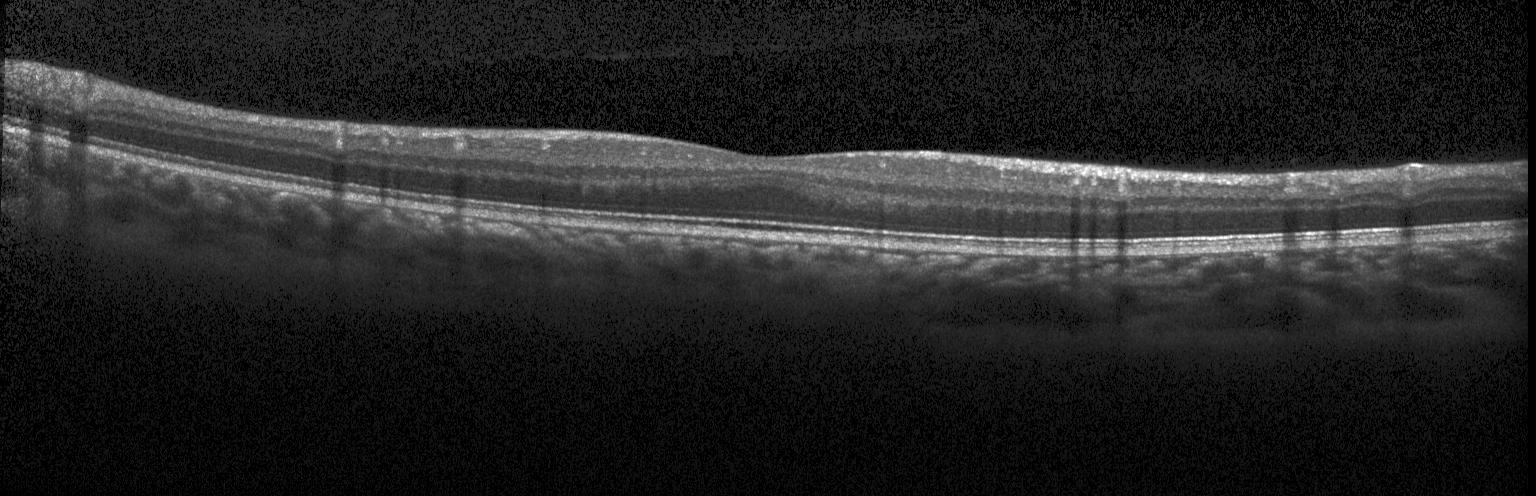

Fovea-centered · retinal OCT cross-section · spectral-domain OCT. Macular OCT: neither CNV, DME, nor drusen.